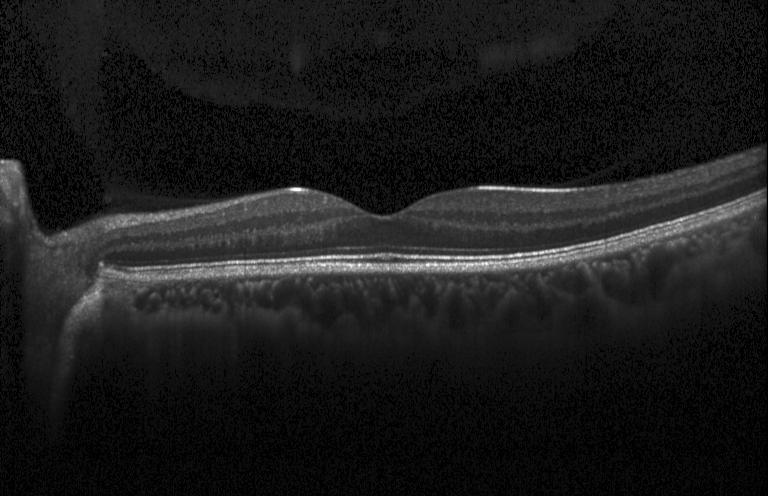

OCT finding: no choroidal neovascularization, no diabetic macular edema, and no drusen.